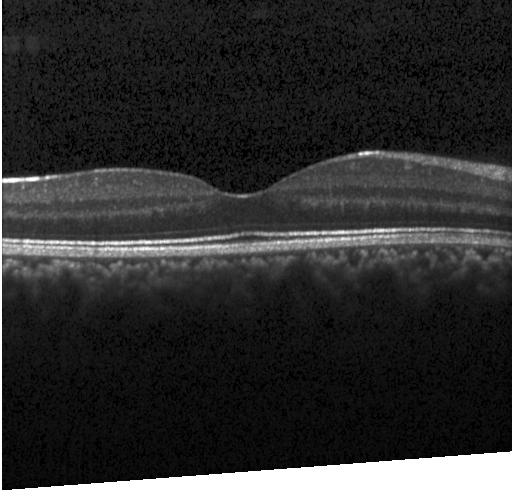 Impression: no choroidal neovascularization, no diabetic macular edema, and no drusen.